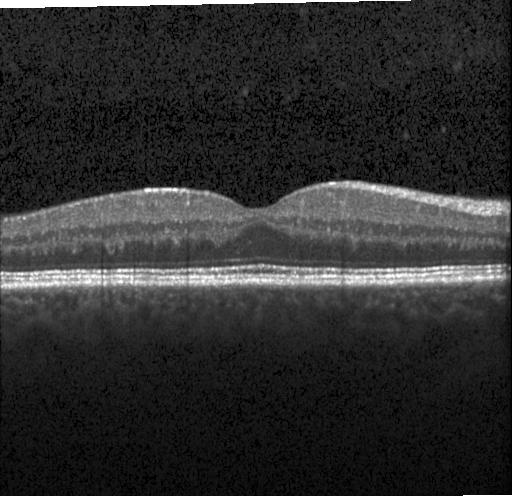 Finding: no evidence of choroidal neovascularization, diabetic macular edema, or drusen.